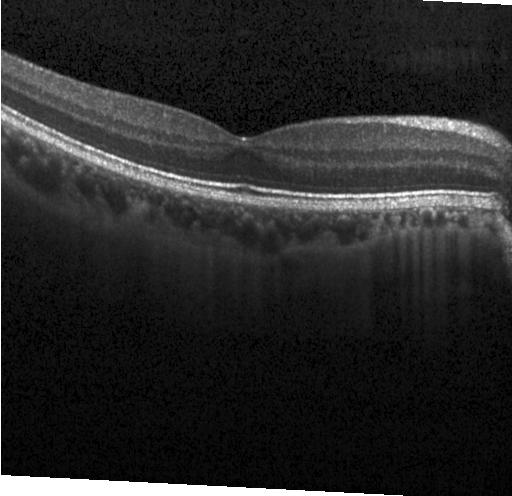

Optical coherence tomography B-scan, macular scan — Diagnosis: no CNV, no DME, and no drusen.